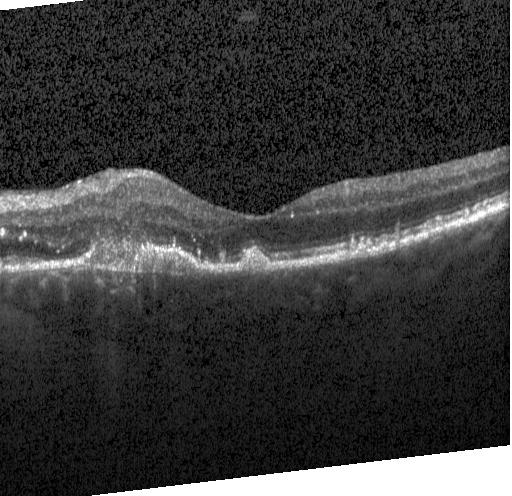
OCT scan showing a choroidal neovascular membrane.